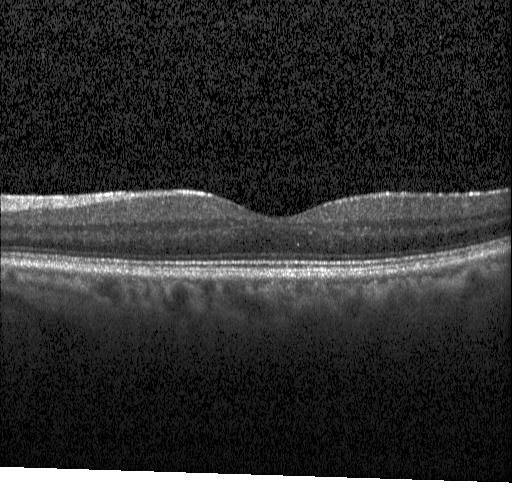
Retinal OCT cross-section · spectral-domain OCT · through the macula · Heidelberg Spectralis
Assessment: no choroidal neovascularization, diabetic macular edema, or drusen.